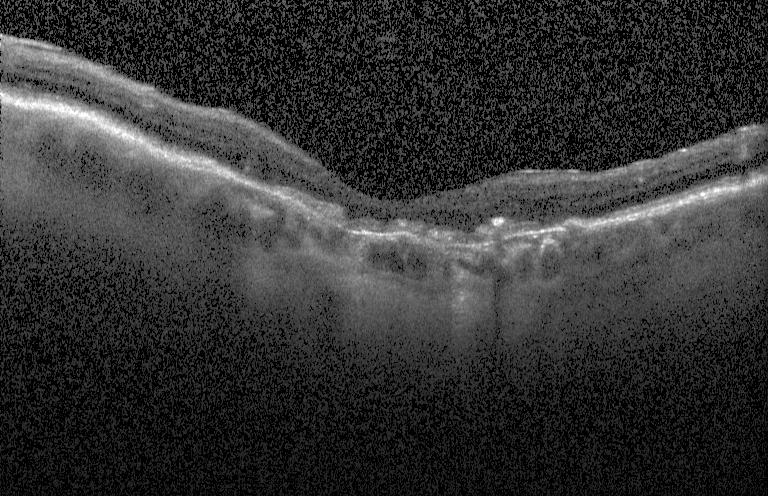

Spectral-domain OCT · optical coherence tomography scan · fovea-centered. Dx: choroidal neovascularization (CNV).